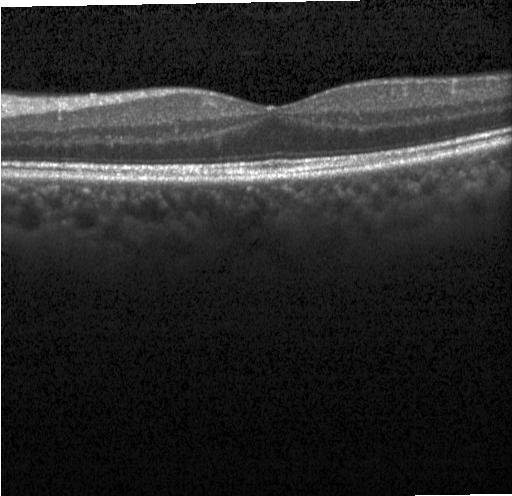
Finding: no evidence of choroidal neovascularization, diabetic macular edema, or drusen.